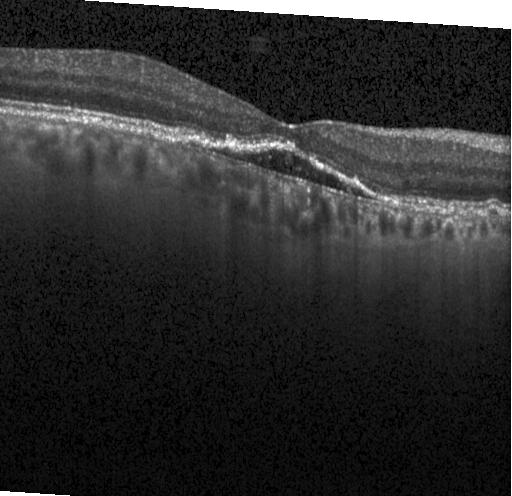

Assessment: choroidal neovascularization.